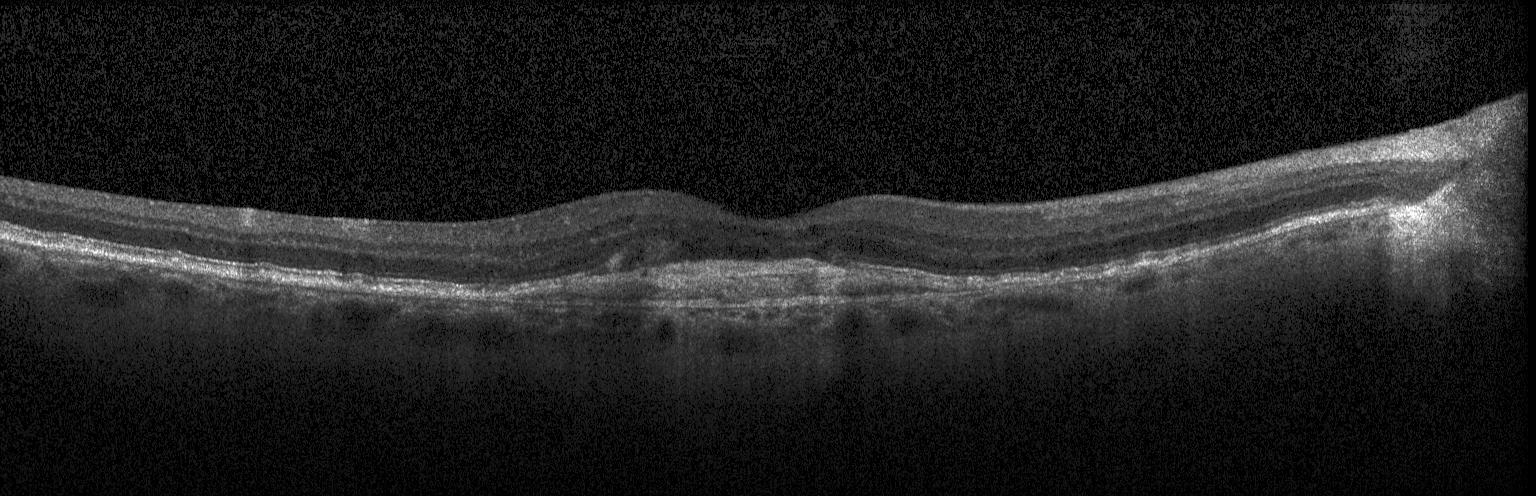 Heidelberg Spectralis OCT system, optical coherence tomography scan, spectral-domain OCT, centered on the fovea
Macular OCT: a choroidal neovascular membrane.